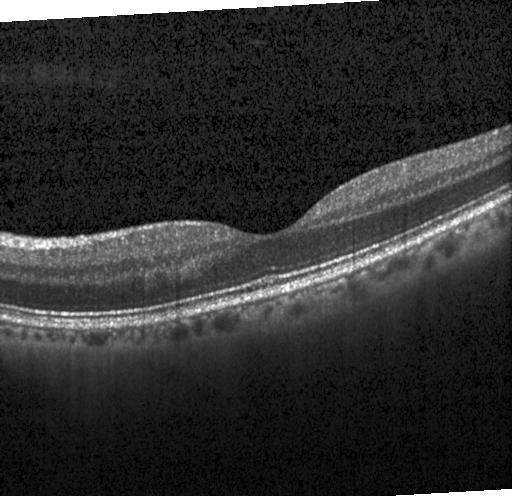
OCT B-scan. Spectral-domain optical coherence tomography. Centered on the fovea
This B-scan demonstrates no evidence of CNV, DME, or drusen.